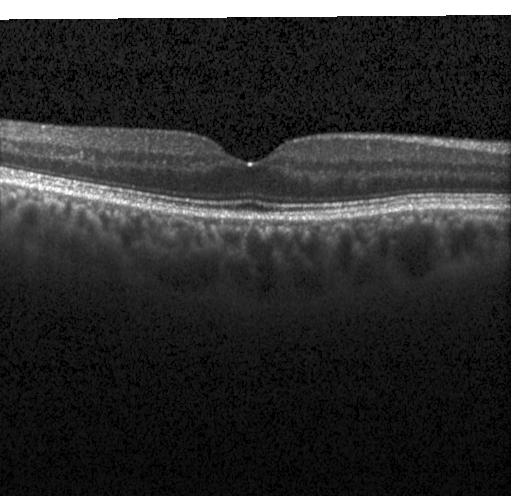
OCT line scan.
Diagnosis: neither CNV, DME, nor drusen.